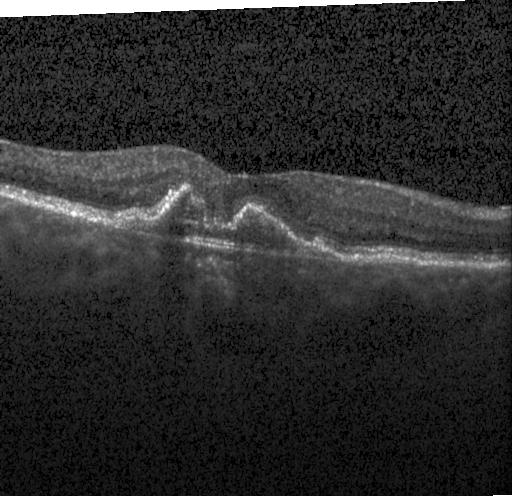 OCT B-scan · centered on the fovea · spectral-domain OCT · instrument: Heidelberg Spectralis. Finding: choroidal neovascularization.